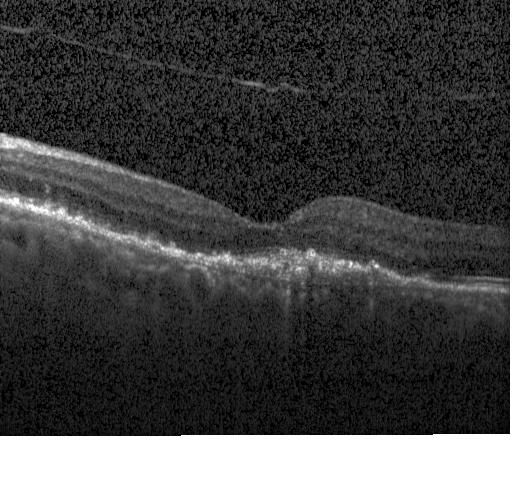 The scan shows choroidal neovascularization (CNV).